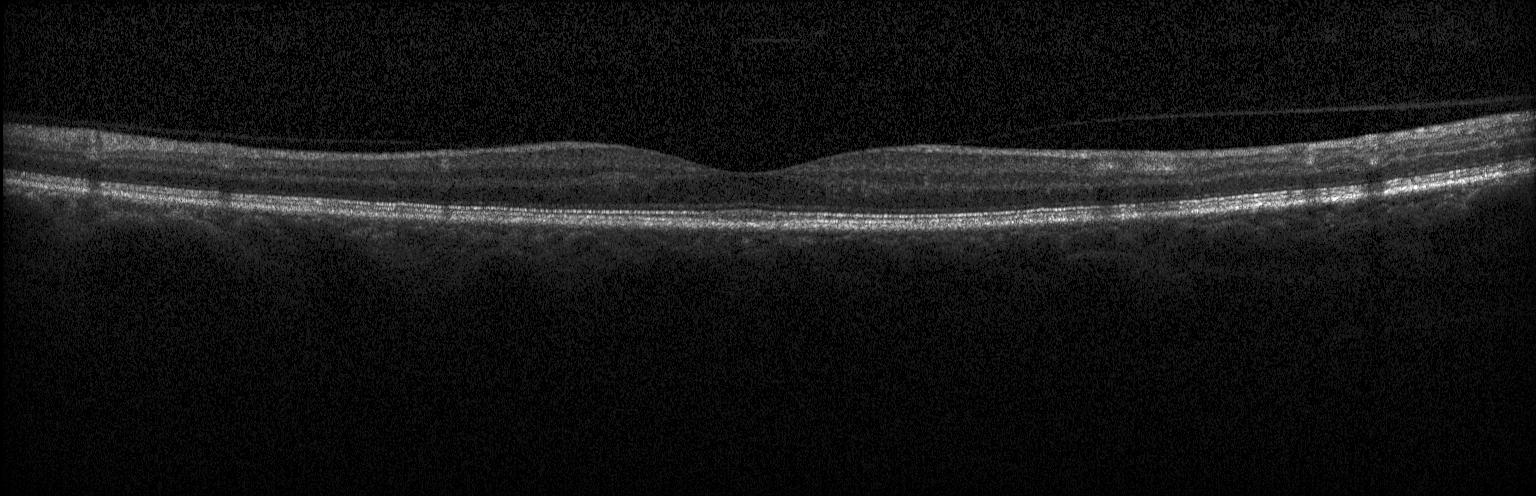

Retinal OCT cross-section showing no CNV, DME, or drusen.